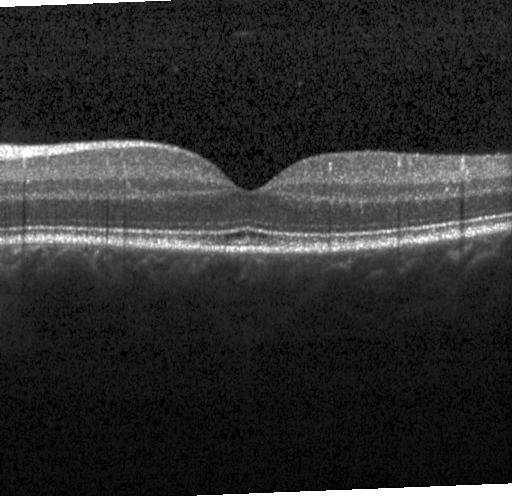 Retinal OCT cross-section showing neither choroidal neovascularization, diabetic macular edema, nor drusen.